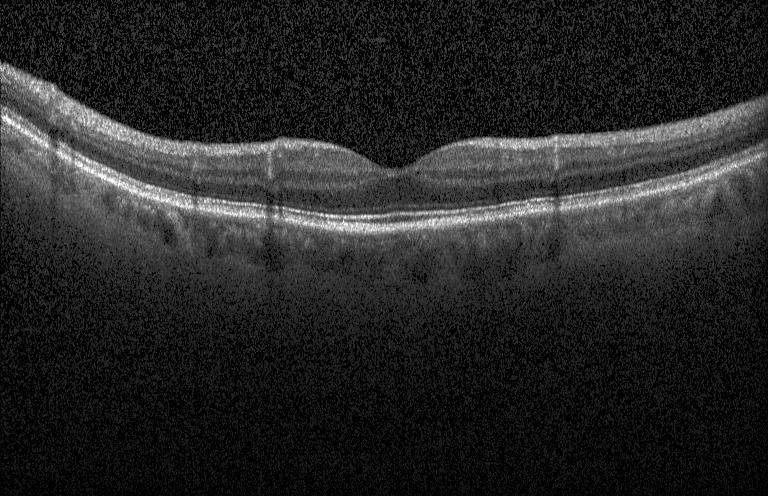
Assessment: no evidence of choroidal neovascularization, diabetic macular edema, or drusen.